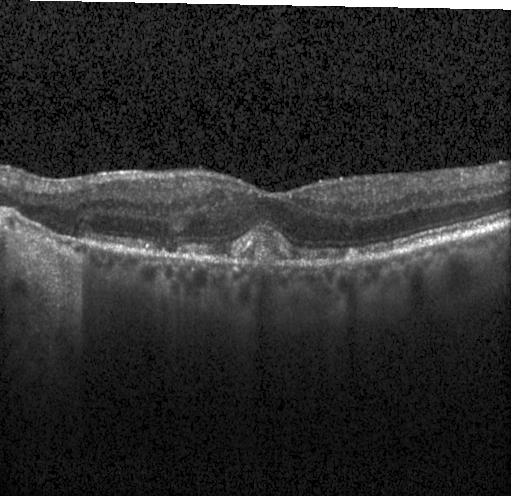

Through the macula · SD-OCT · optical coherence tomography B-scan · Heidelberg Spectralis.
Dx: a choroidal neovascular membrane.